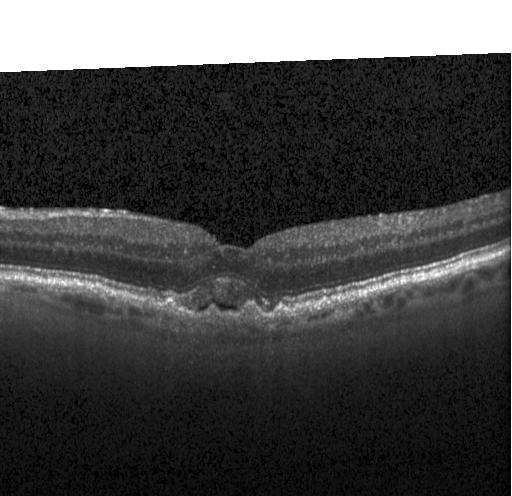

OCT B-scan; centered on the fovea; acquired on a Heidelberg Spectralis — OCT finding: a choroidal neovascular membrane.